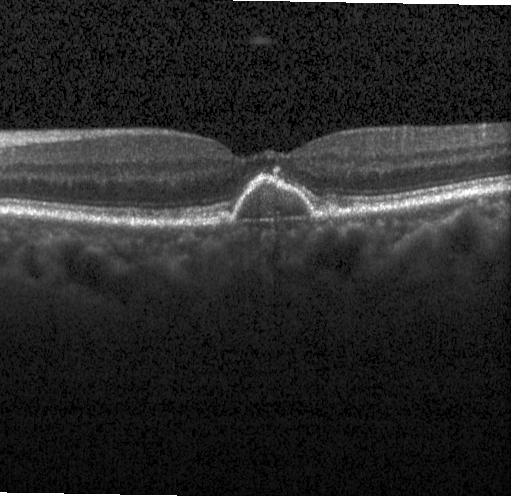

Centered on the fovea · OCT B-scan · instrument: Heidelberg Spectralis · spectral-domain optical coherence tomography.
Diagnosis: a choroidal neovascular membrane.